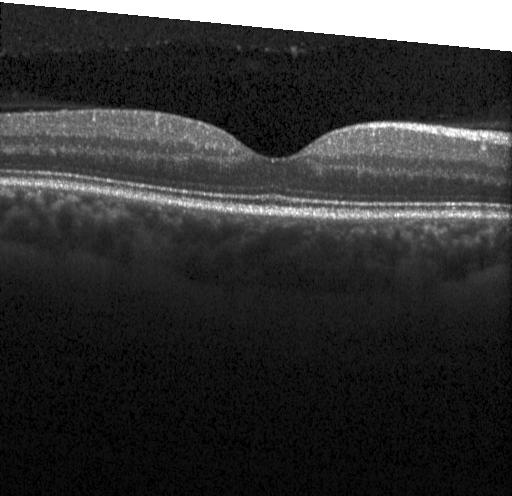
Optical coherence tomography scan · Heidelberg Spectralis OCT system · macular scan.
OCT finding: no choroidal neovascularization, diabetic macular edema, or drusen.